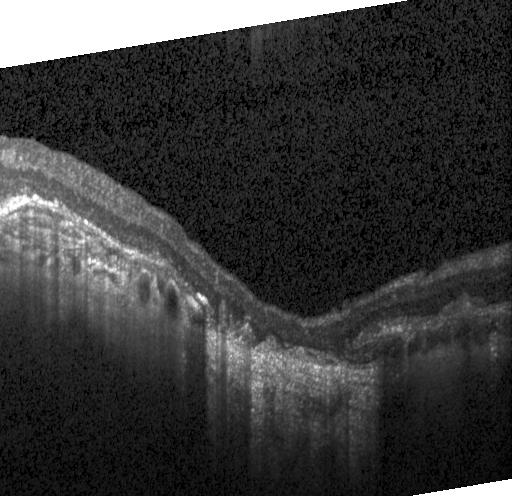

Macular OCT: choroidal neovascularization.